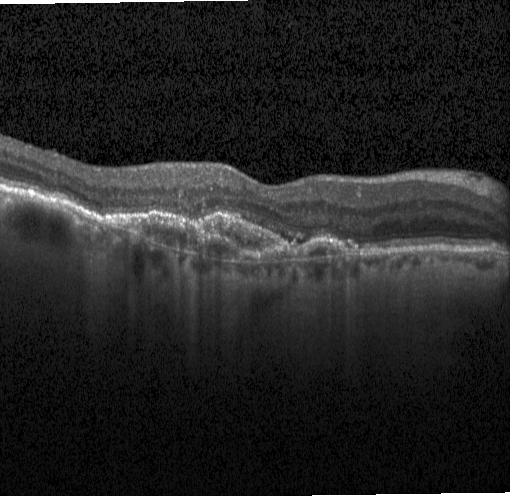
Dx: a choroidal neovascular membrane.